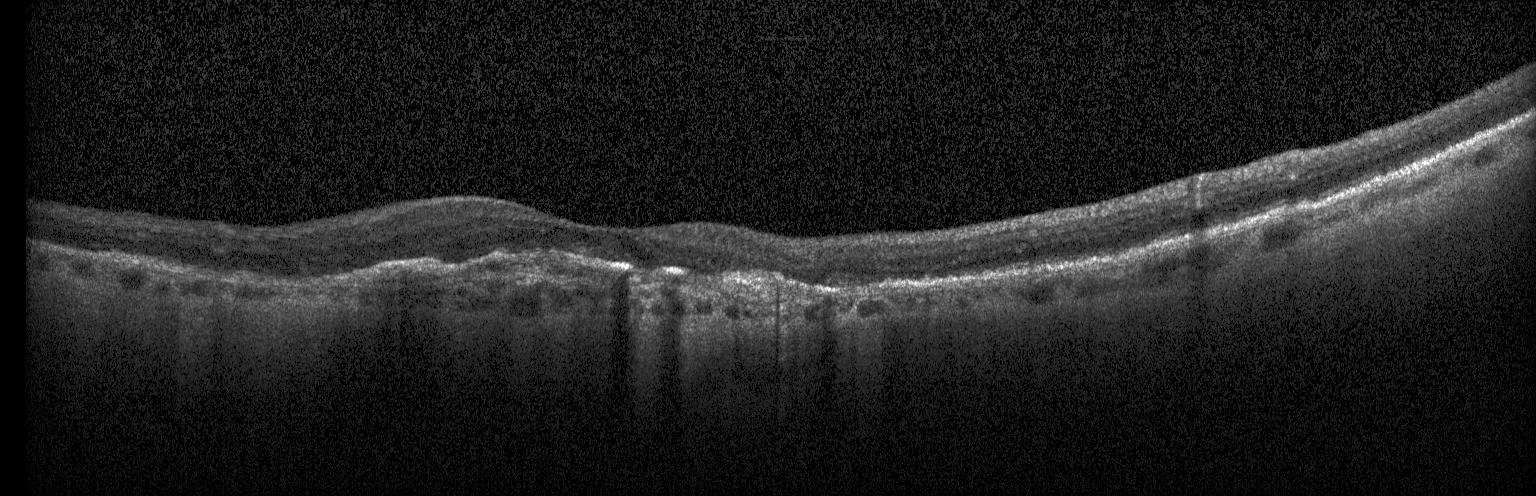

OCT line scan. This B-scan demonstrates choroidal neovascularization.